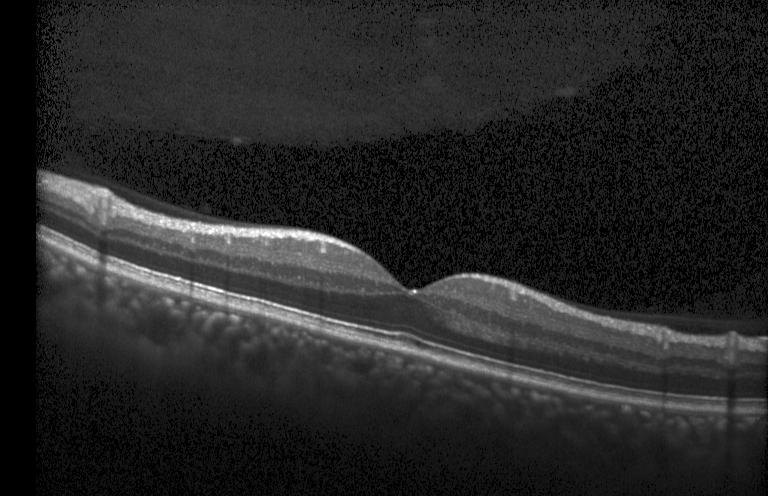

Impression: neither choroidal neovascularization, diabetic macular edema, nor drusen.